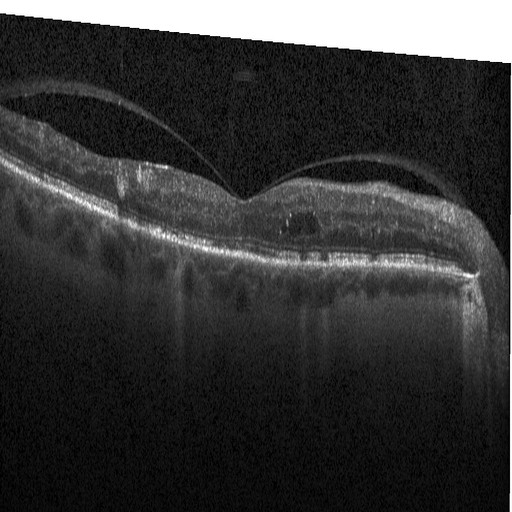 Through the macula. Spectral-domain optical coherence tomography. Instrument: Heidelberg Spectralis. OCT B-scan — OCT finding: DME.